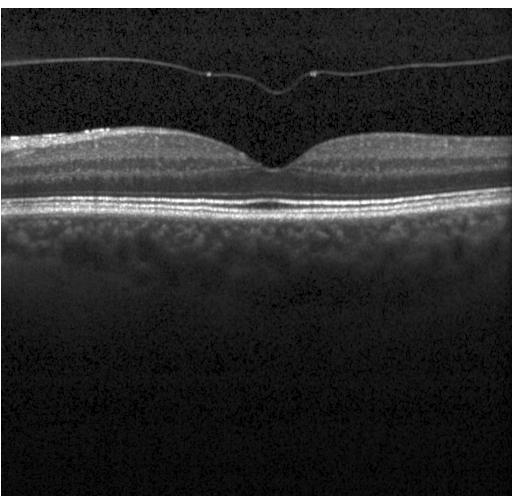

Optical coherence tomography B-scan. Impression: neither choroidal neovascularization, diabetic macular edema, nor drusen.